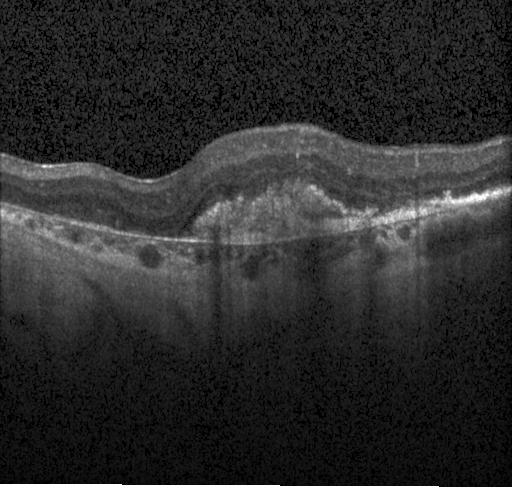 Retinal OCT cross-section.
Finding: choroidal neovascularization.